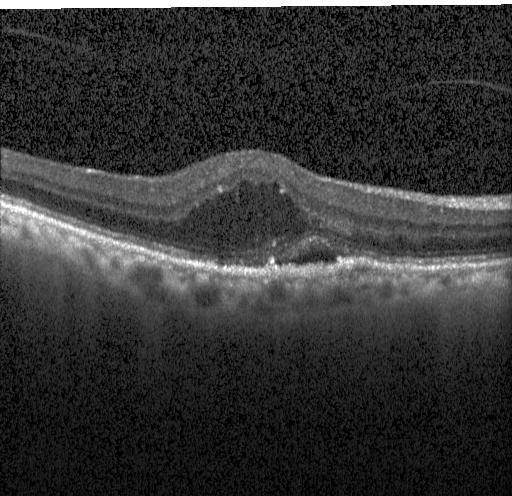 Retinal OCT cross-section
A choroidal neovascular membrane.